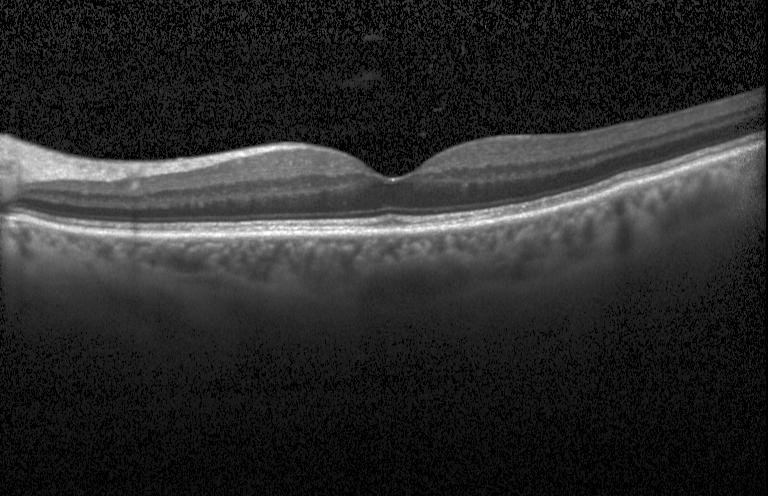 Impression: no choroidal neovascularization, no diabetic macular edema, and no drusen.